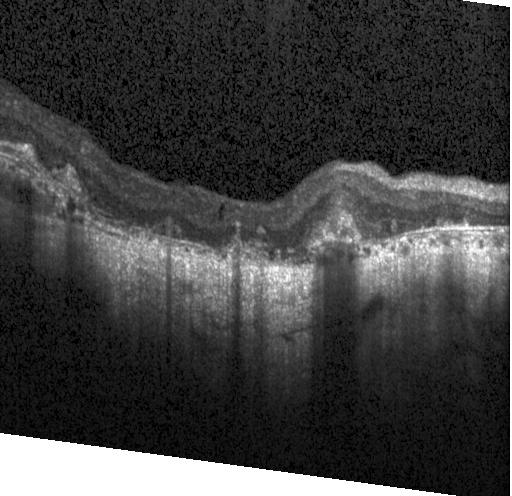 Impression: choroidal neovascularization (CNV).